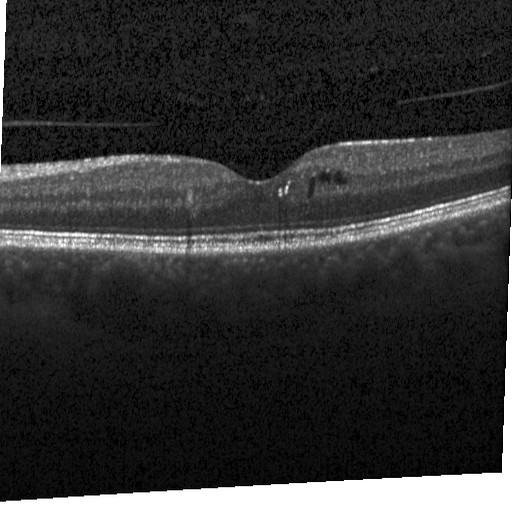 Acquired on a Heidelberg Spectralis, optical coherence tomography scan
Assessment: diabetic macular edema (DME).